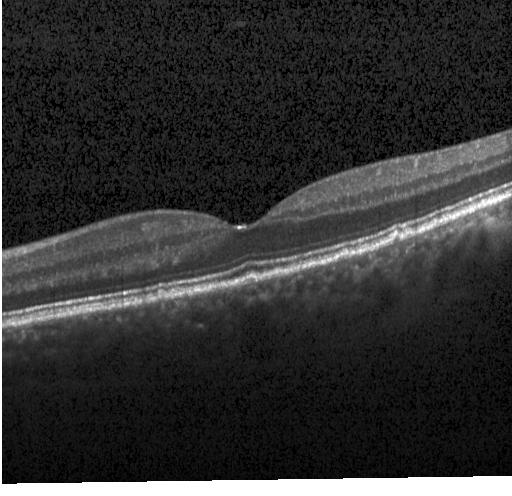 OCT line scan. Centered on the fovea. SD-OCT. Acquired on a Heidelberg Spectralis
Finding: drusen.